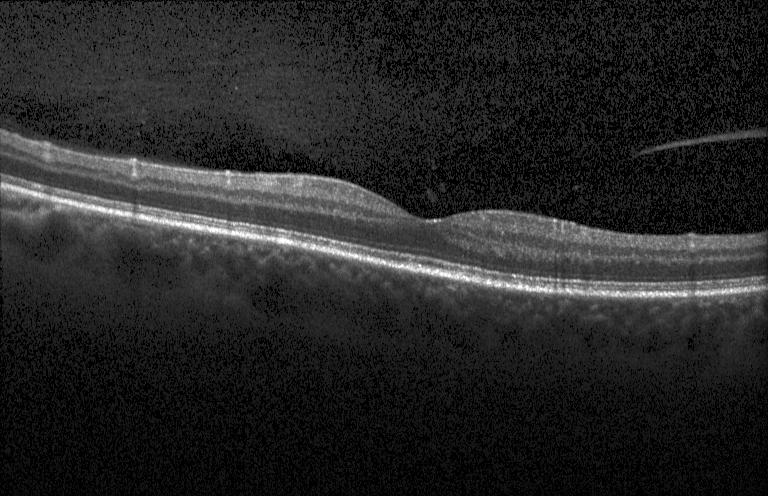

Optical coherence tomography B-scan. Acquired on a Heidelberg Spectralis. Spectral-domain optical coherence tomography — The scan shows no choroidal neovascularization, no diabetic macular edema, and no drusen.